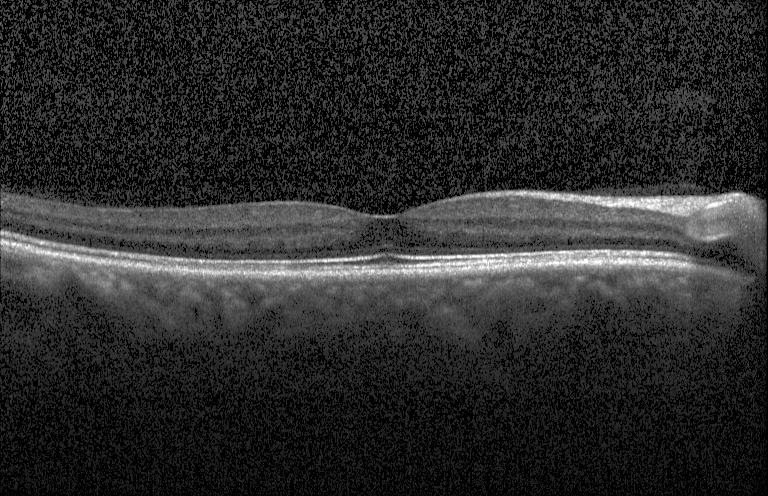 OCT B-scan. Diagnosis: no choroidal neovascularization, diabetic macular edema, or drusen.